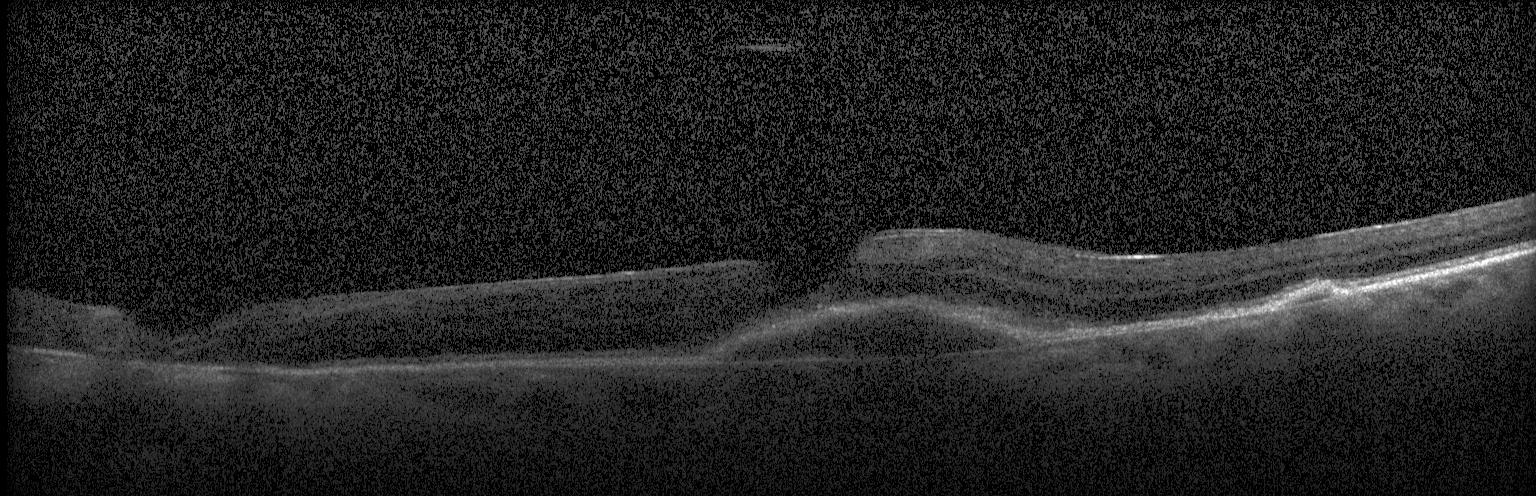 Spectral-domain OCT. Heidelberg Spectralis OCT system. Centered on the fovea. Retinal OCT cross-section.
Finding: a choroidal neovascular membrane.